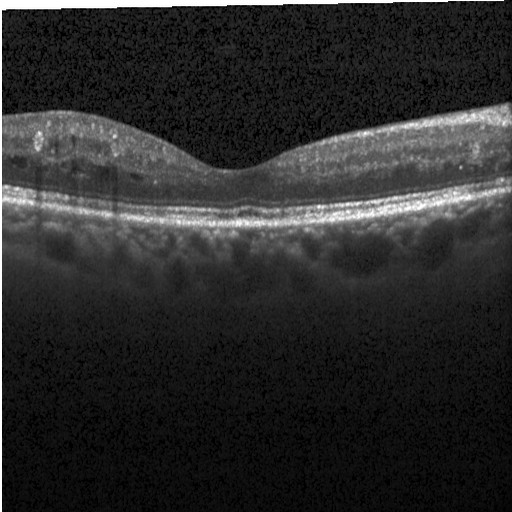 OCT finding: diabetic macular edema.